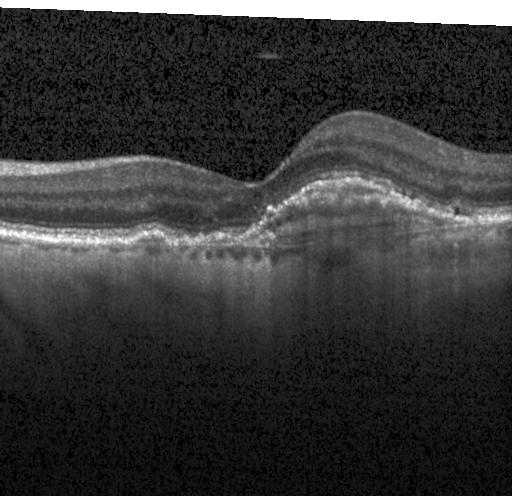
This B-scan demonstrates a choroidal neovascular membrane.